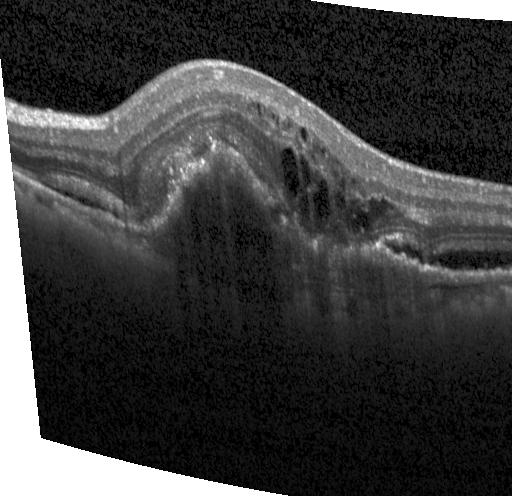 Optical coherence tomography scan. Instrument: Heidelberg Spectralis. Finding: a choroidal neovascular membrane.